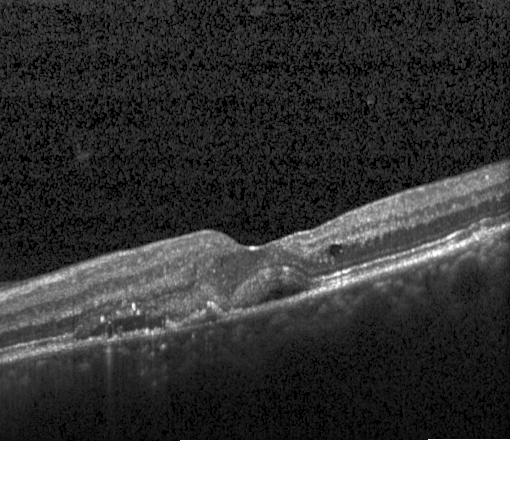
Retinal OCT B-scan. Heidelberg Spectralis — Impression: a choroidal neovascular membrane.